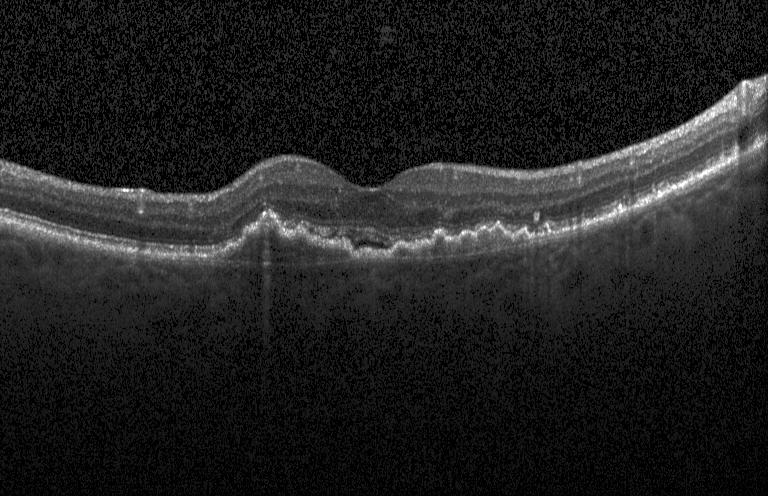

Spectral-domain OCT B-scan: choroidal neovascularization (CNV).